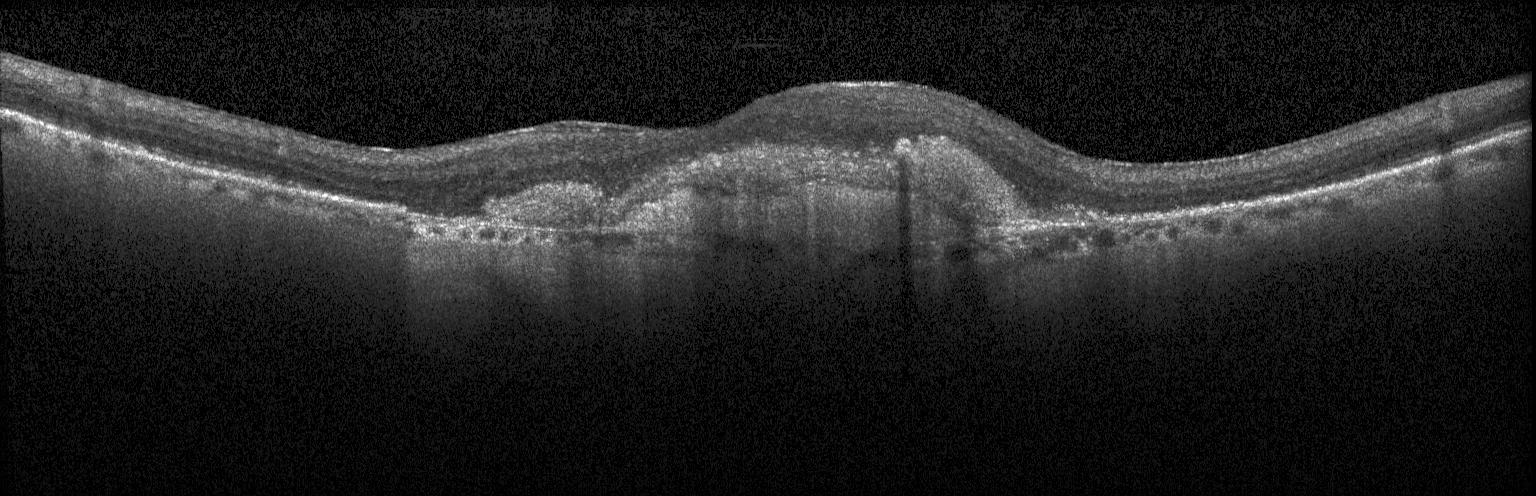

Spectral-domain OCT B-scan: a choroidal neovascular membrane.